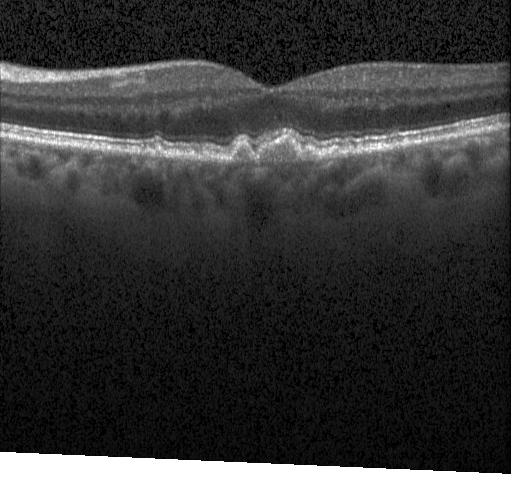 Optical coherence tomography scan. Spectral-domain optical coherence tomography. Through the macula
Diagnosis: drusen.